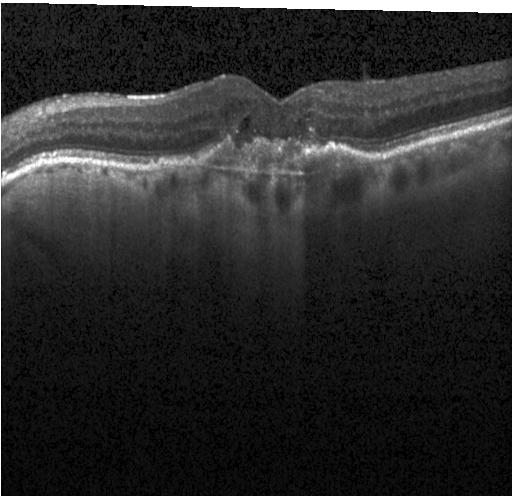
Heidelberg Spectralis OCT system; retinal OCT cross-section. Impression: a choroidal neovascular membrane.